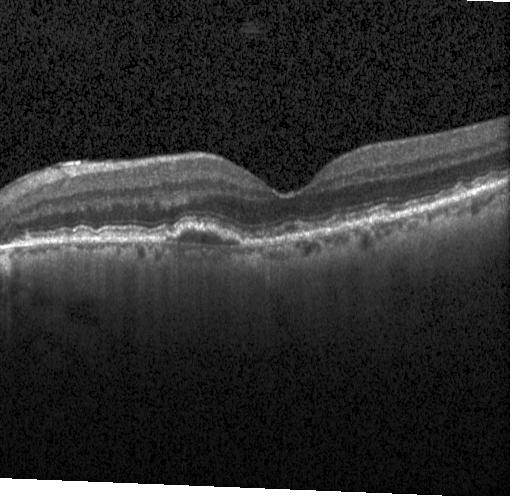 Optical coherence tomography scan. Spectral-domain optical coherence tomography. Macular scan.
Assessment: a choroidal neovascular membrane.